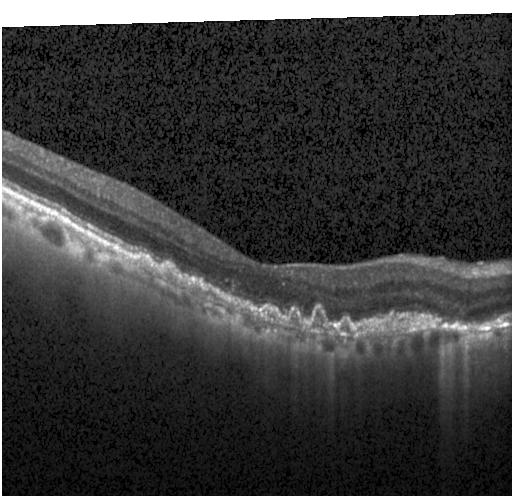

Retinal OCT B-scan — Finding: a choroidal neovascular membrane.